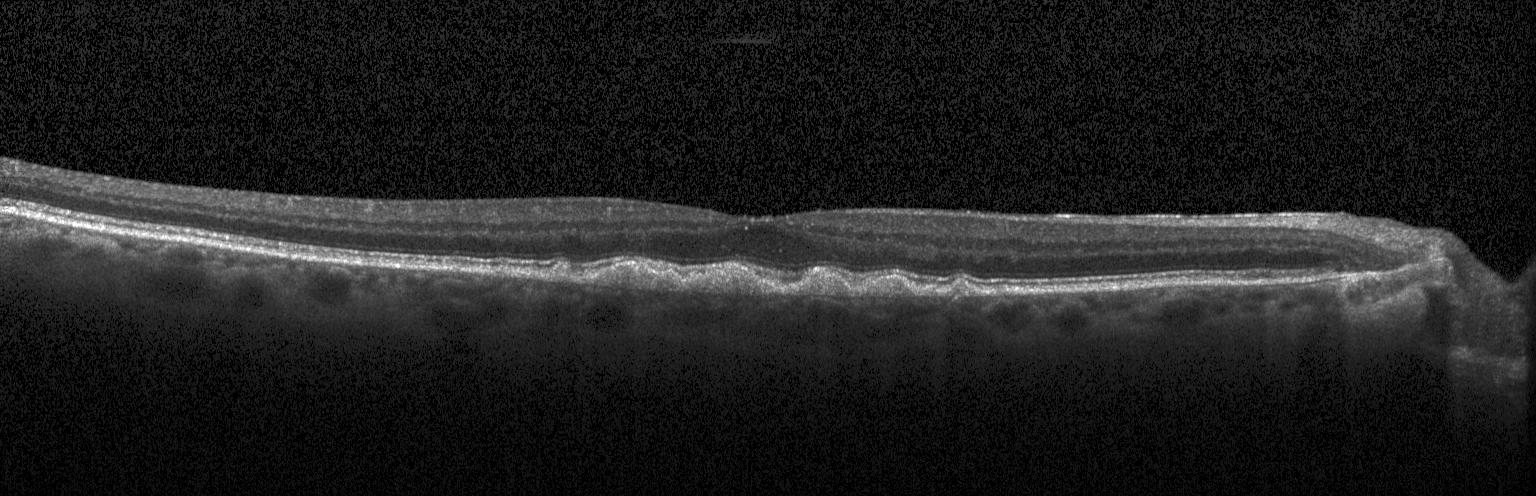
Retinal OCT cross-section — Drusen.